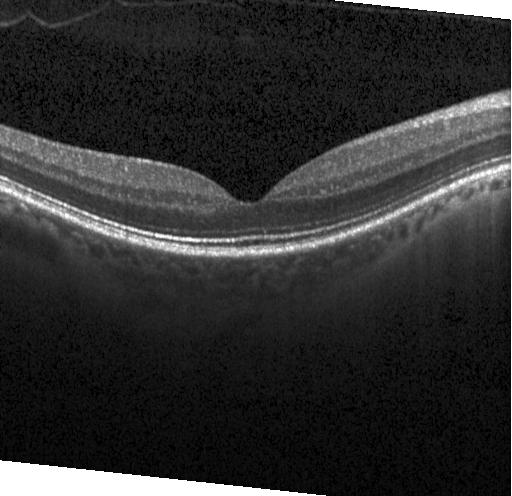

Optical coherence tomography scan — Finding: neither choroidal neovascularization, diabetic macular edema, nor drusen.